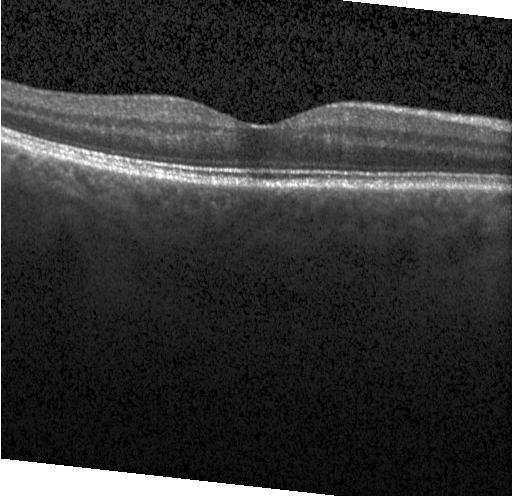
OCT finding: no evidence of choroidal neovascularization, diabetic macular edema, or drusen.